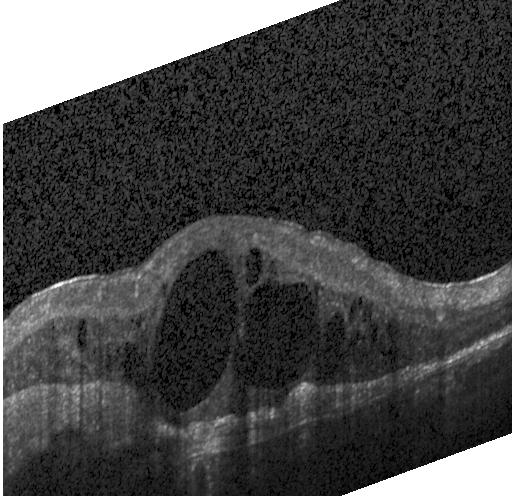
Retinal OCT cross-section; instrument: Heidelberg Spectralis; horizontal scan through the fovea
This B-scan demonstrates CNV.